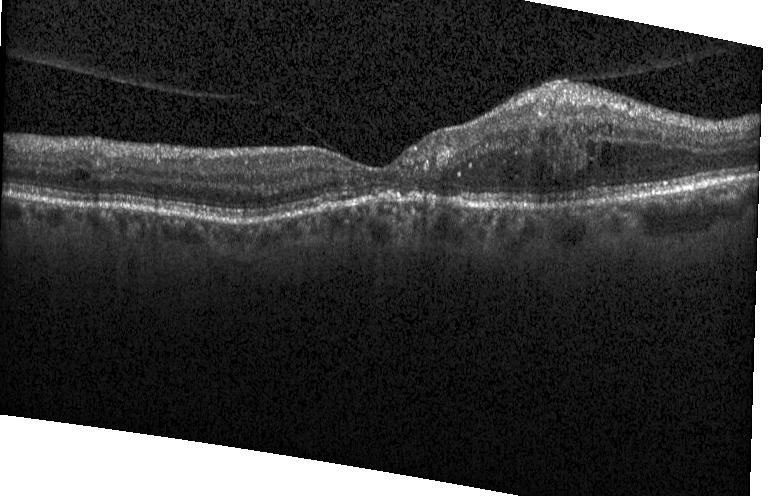

Diagnosis: CNV.